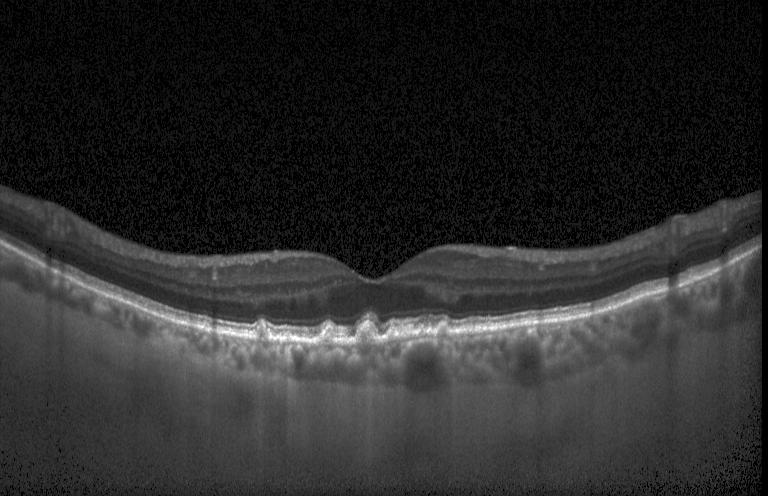

Macular scan; OCT B-scan — Finding: multiple drusen.